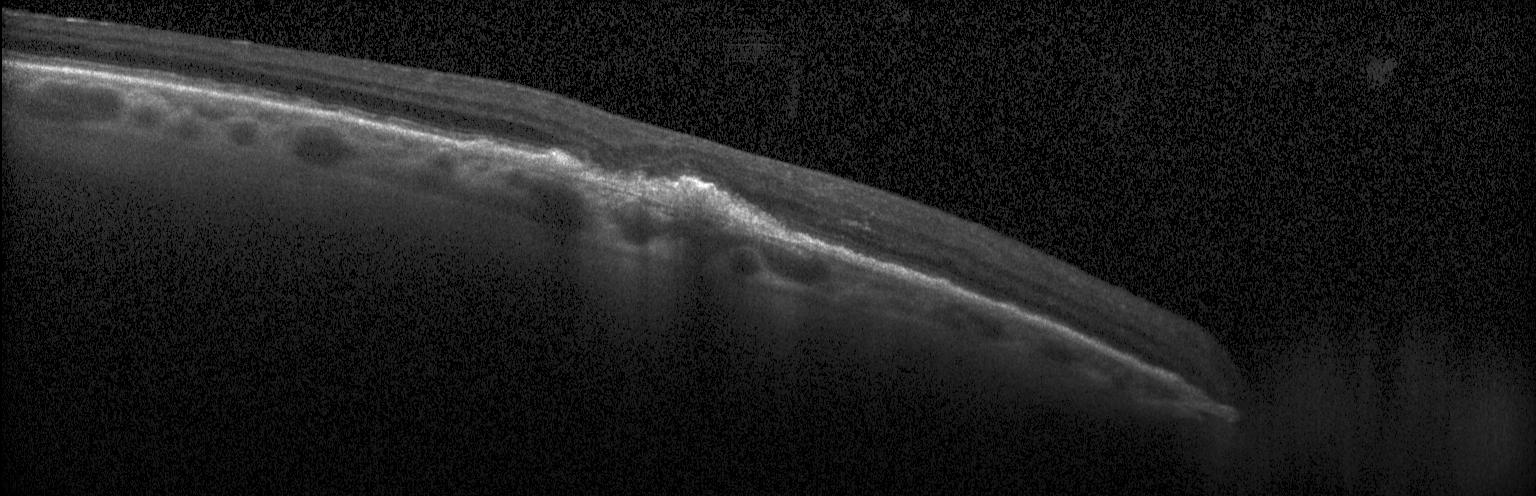 Assessment: choroidal neovascularization (CNV).